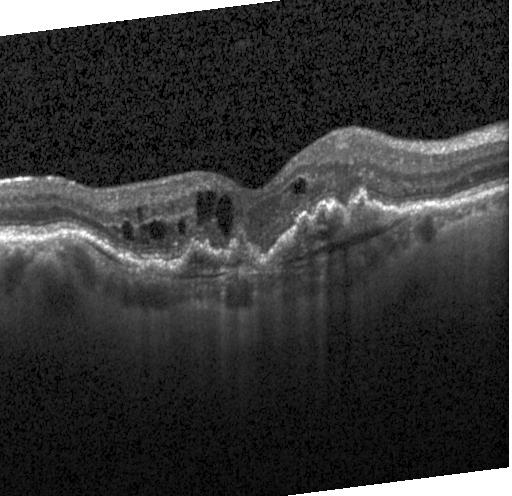 OCT finding: CNV.